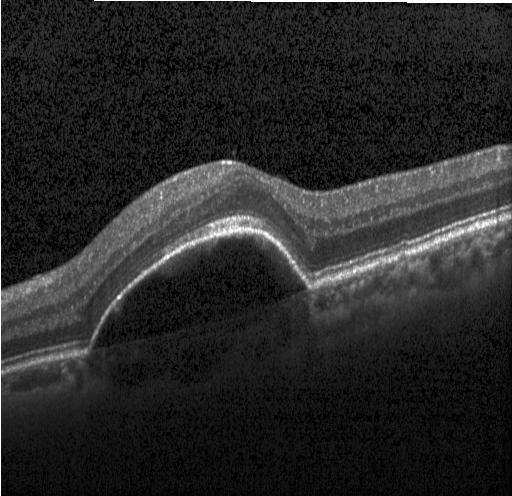 Impression: a choroidal neovascular membrane.